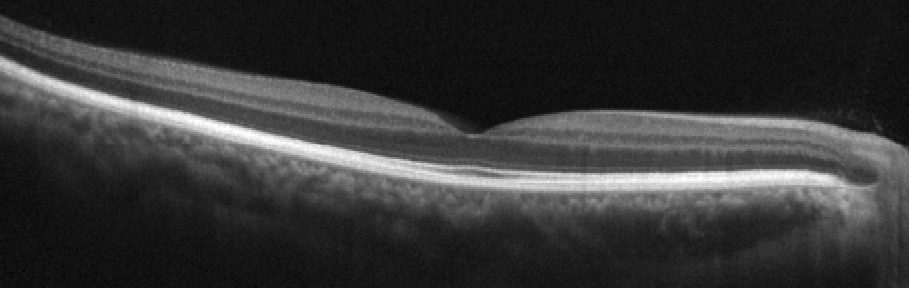
Instrument: Optovue Avanti RTVue XR · macular scan · retinal OCT cross-section
No evidence of AMD, DME, ERM, RAO, RVO, or VID.